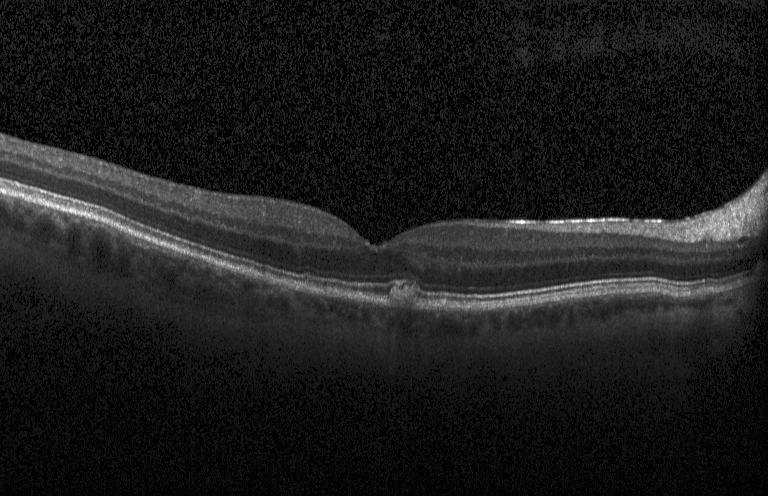
Impression: drusen.